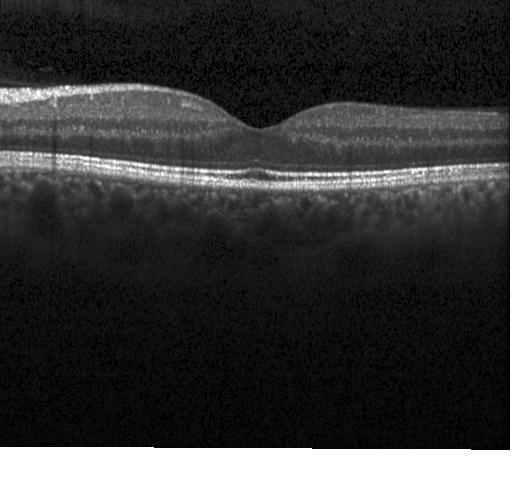
Finding: no evidence of choroidal neovascularization, diabetic macular edema, or drusen.